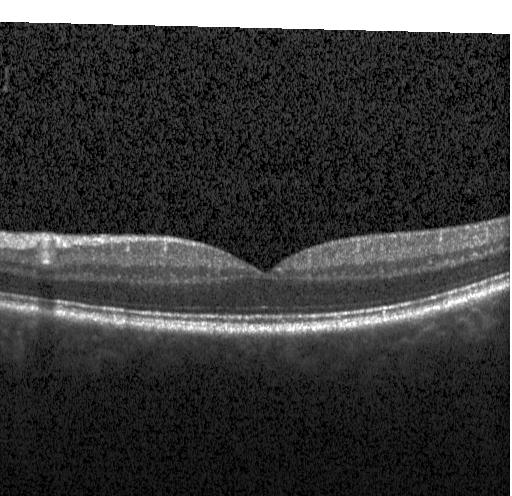

The scan shows no choroidal neovascularization, no diabetic macular edema, and no drusen.